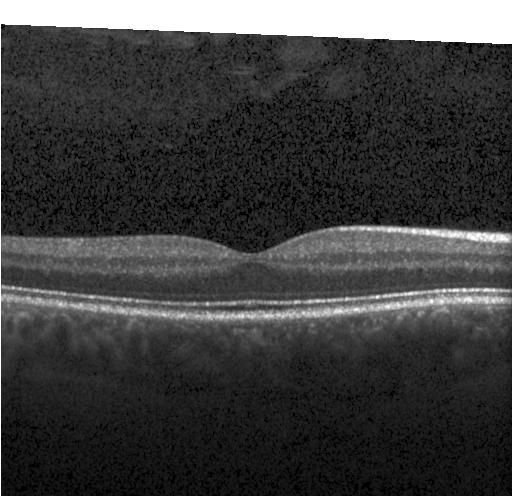

Heidelberg Spectralis. Fovea-centered. Optical coherence tomography scan. Spectral-domain OCT
Impression: no evidence of choroidal neovascularization, diabetic macular edema, or drusen.